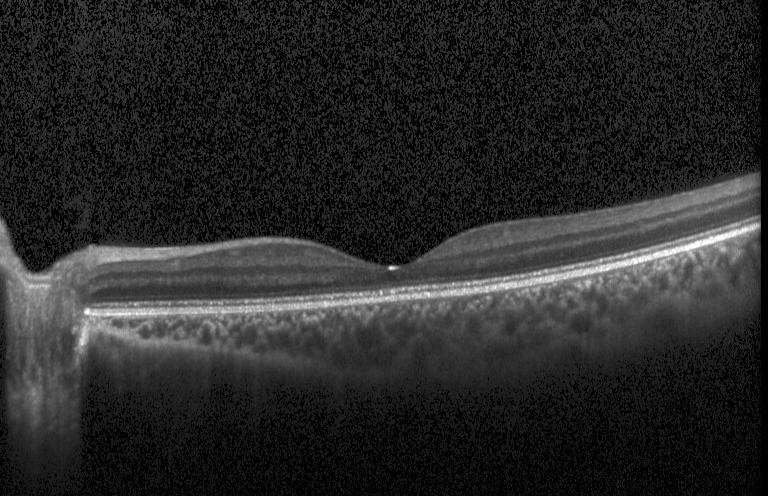
Dx: no choroidal neovascularization, no diabetic macular edema, and no drusen.